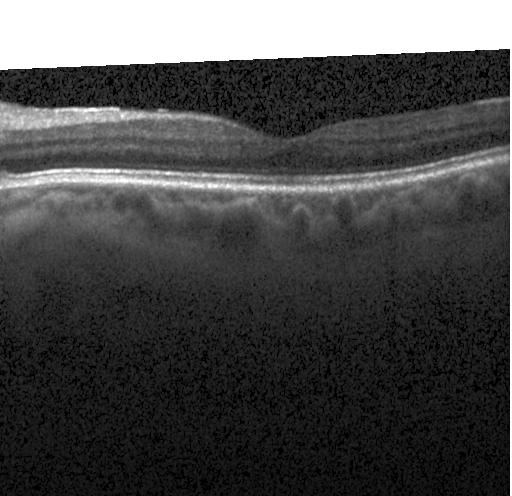

Heidelberg Spectralis. Retinal OCT B-scan — This B-scan demonstrates neither choroidal neovascularization, diabetic macular edema, nor drusen.